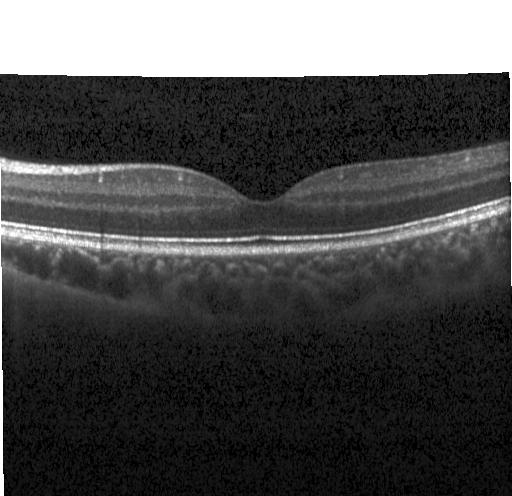

OCT B-scan
Impression: neither choroidal neovascularization, diabetic macular edema, nor drusen.